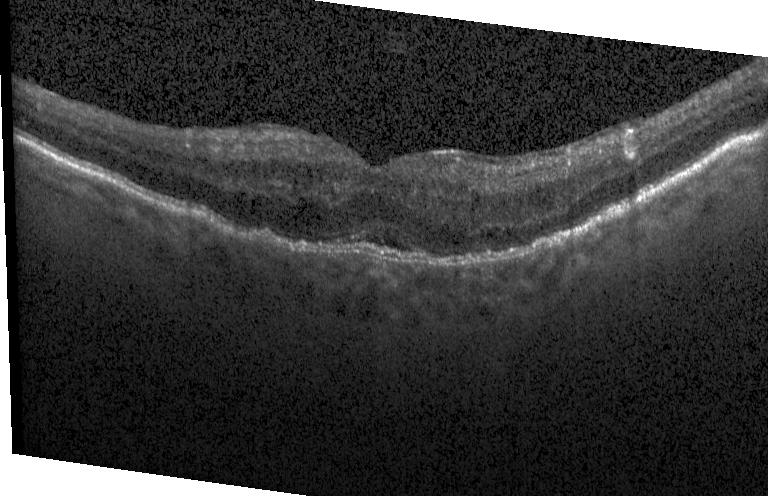 OCT B-scan showing choroidal neovascularization (CNV).